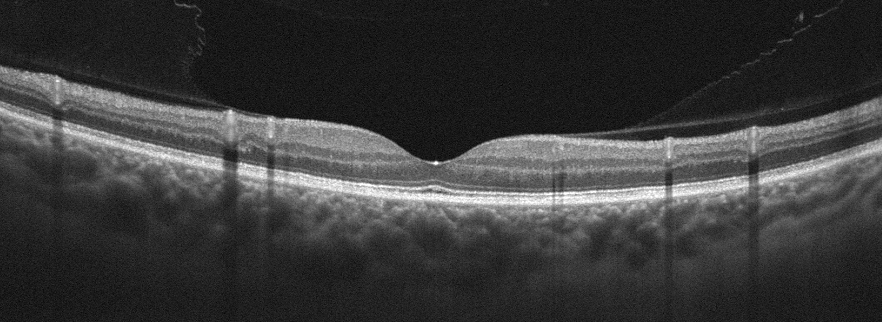 Optical coherence tomography B-scan, Optovue Avanti RTVue XR, macular scan, left eye. This B-scan demonstrates no AMD, DME, ERM, RAO, RVO, or VID.